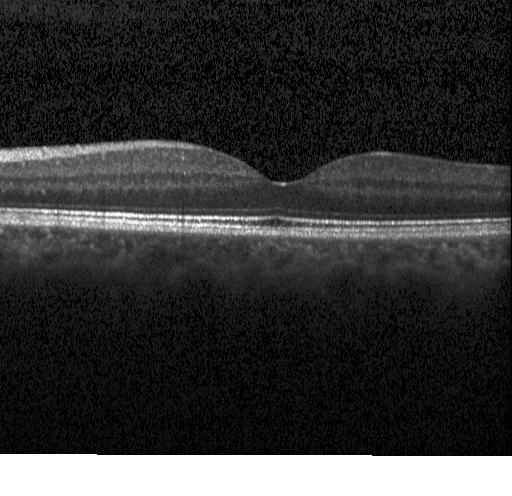 OCT B-scan · through the macula — Macular OCT: no choroidal neovascularization, diabetic macular edema, or drusen.